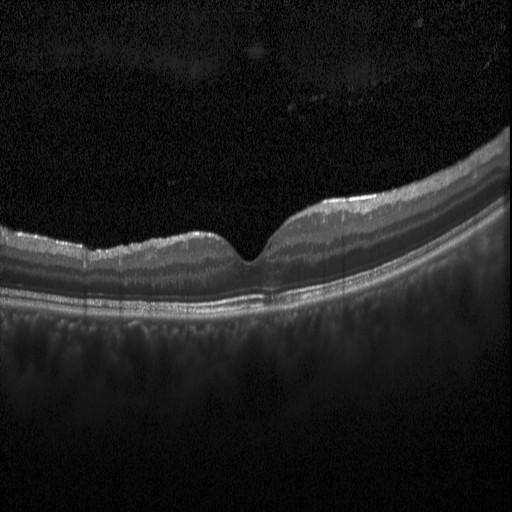
Fovea-centered; retinal OCT B-scan; spectral-domain OCT. Macular OCT: diabetic macular edema.